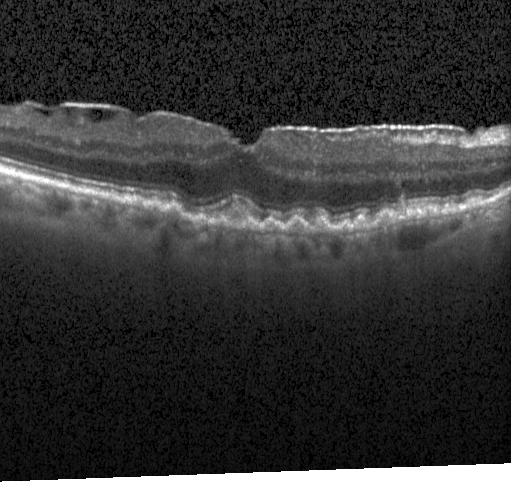 Retinal OCT B-scan · acquired on a Heidelberg Spectralis · macular scan — Macular OCT: multiple drusen.